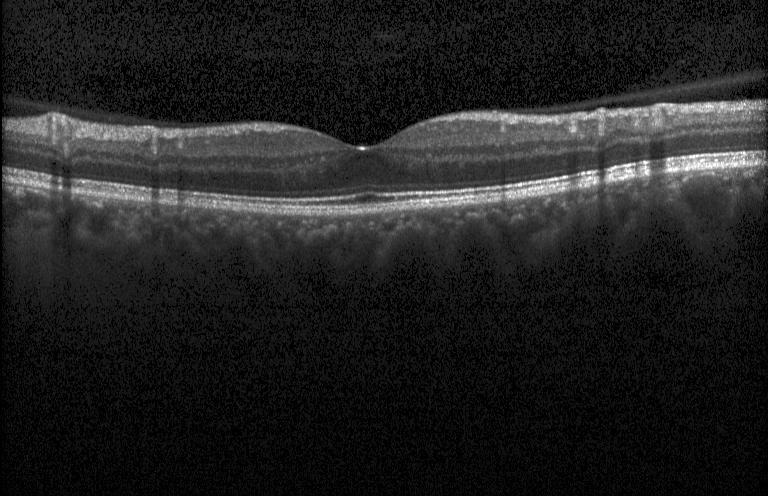
Spectral-domain OCT. OCT line scan. Macular scan. Heidelberg Spectralis
Finding: no evidence of choroidal neovascularization, diabetic macular edema, or drusen.